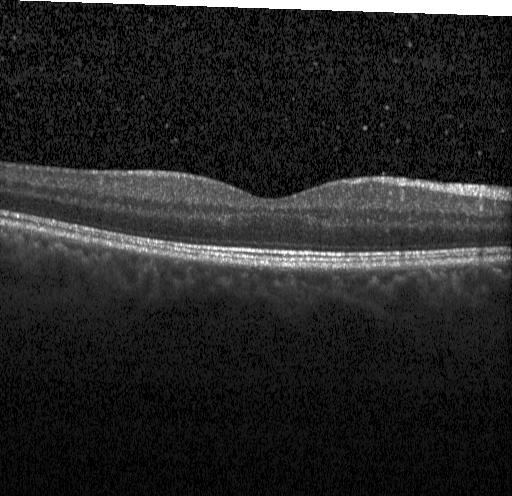

OCT B-scan; spectral-domain optical coherence tomography; fovea-centered
Assessment: no CNV, no DME, and no drusen.